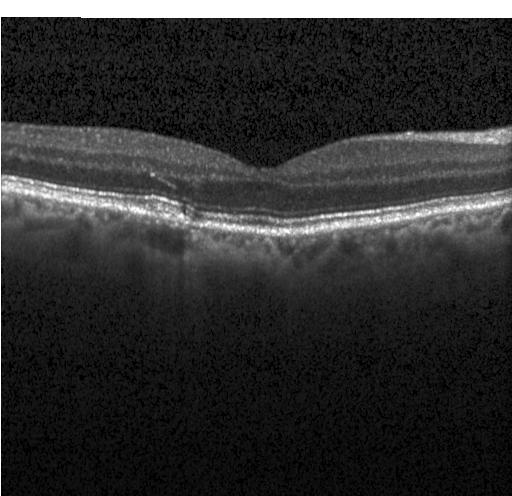 Retinal OCT cross-section.
Diagnosis: sub-RPE drusenoid deposits.